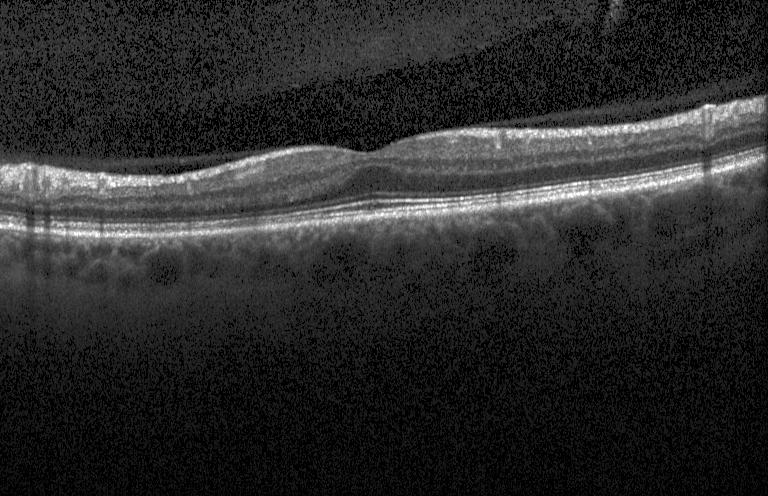

Spectral-domain OCT B-scan: no choroidal neovascularization, diabetic macular edema, or drusen.